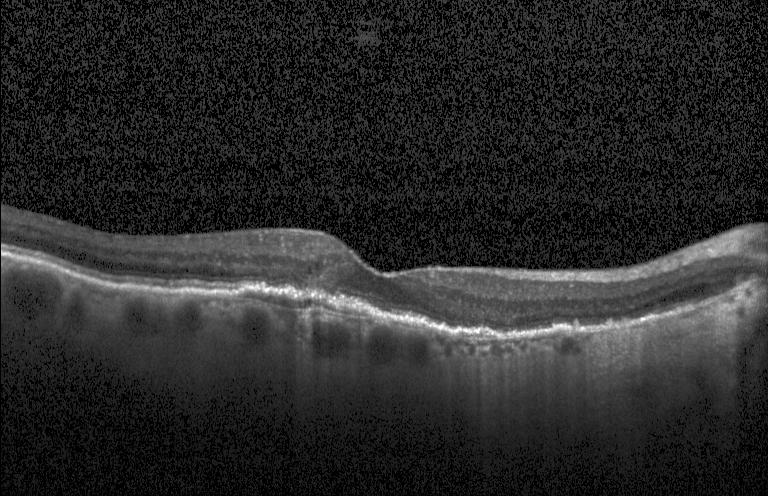

Assessment: CNV.